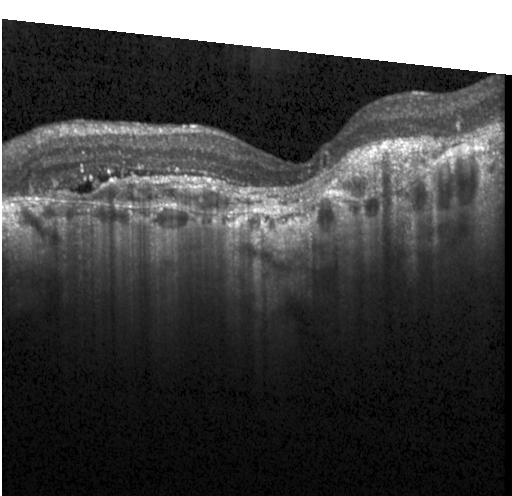
Finding: choroidal neovascularization.